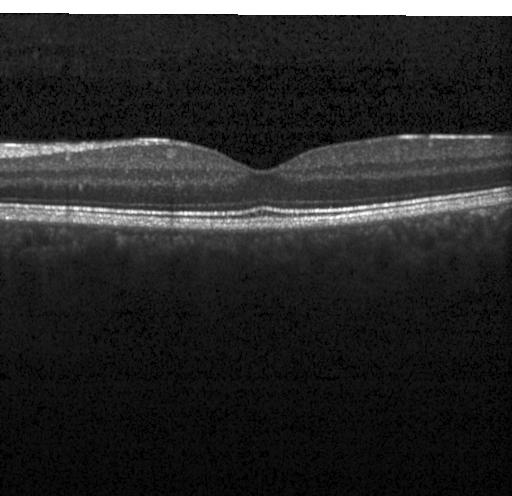
Spectral-domain OCT, OCT line scan, fovea-centered.
The scan shows neither choroidal neovascularization, diabetic macular edema, nor drusen.